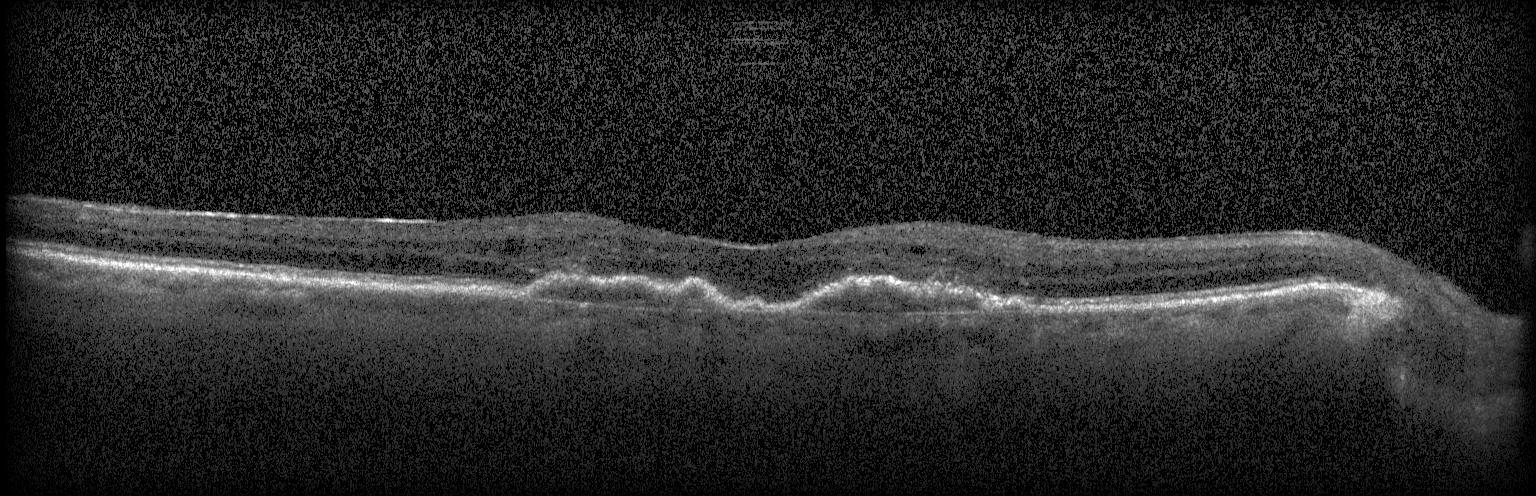
Diagnosis: choroidal neovascularization (CNV).